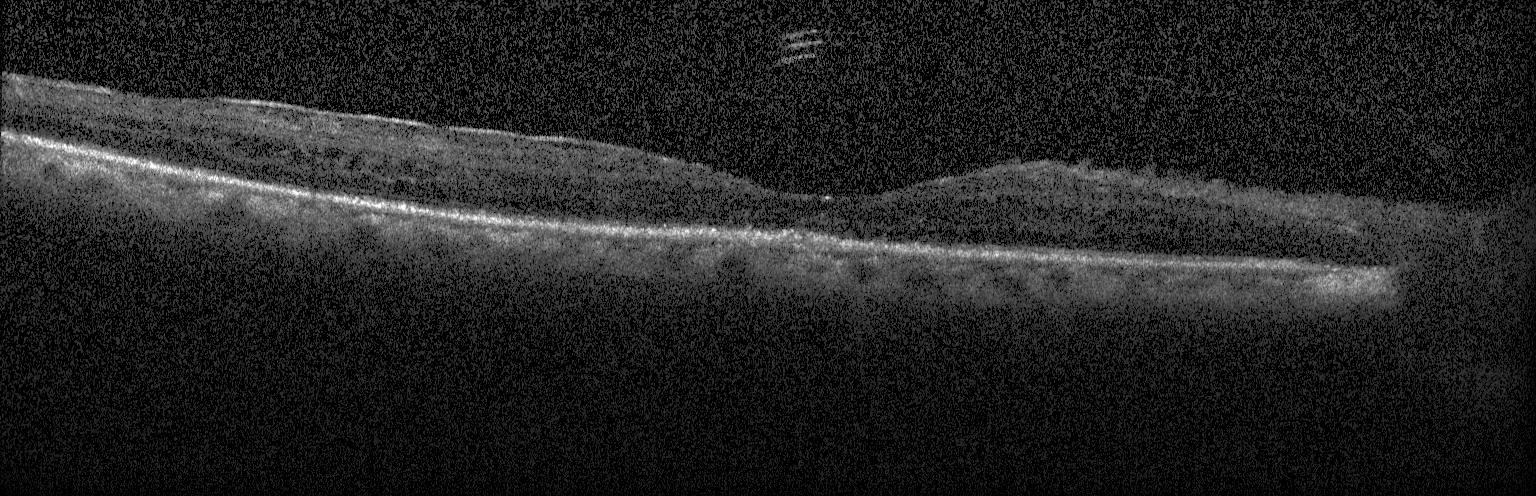
OCT B-scan. Spectral-domain OCT. Horizontal scan through the fovea — Assessment: diabetic macular edema.